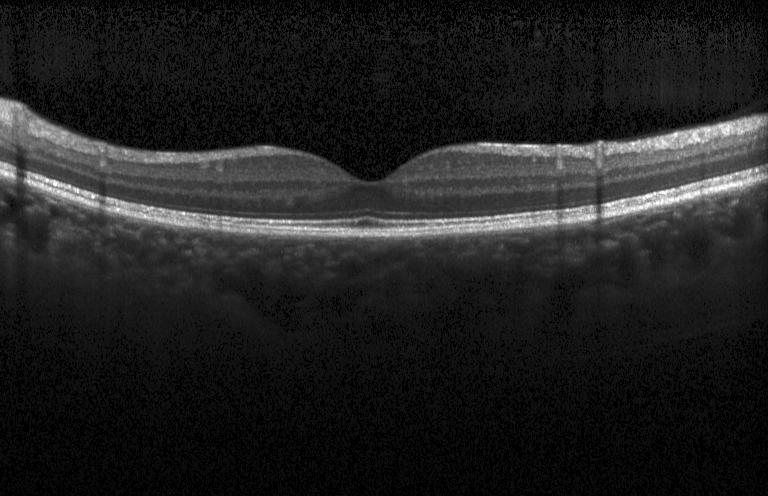

Instrument: Heidelberg Spectralis, optical coherence tomography scan, macular scan, spectral-domain OCT.
Diagnosis: no evidence of choroidal neovascularization, diabetic macular edema, or drusen.